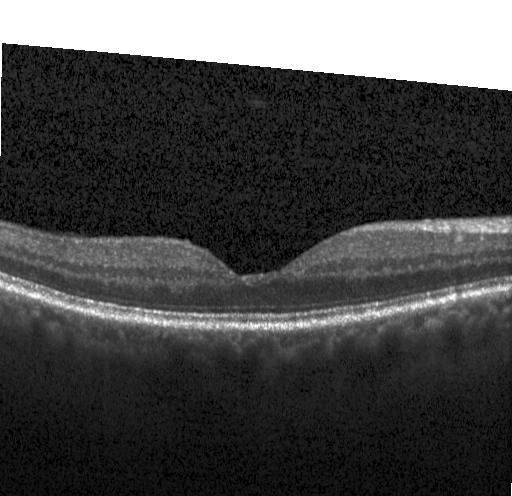

Heidelberg Spectralis, retinal OCT B-scan
Impression: no choroidal neovascularization, no diabetic macular edema, and no drusen.